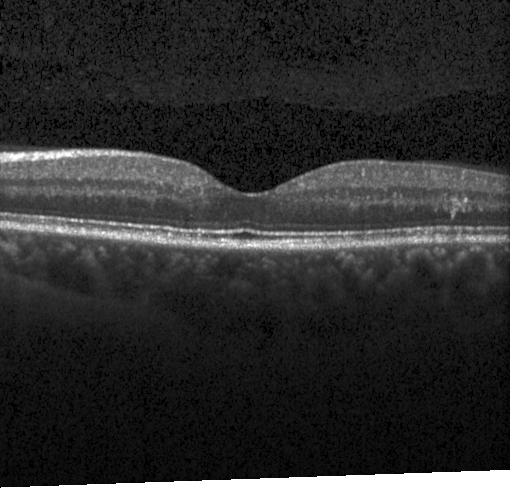
Spectral-domain optical coherence tomography, centered on the fovea, acquired on a Heidelberg Spectralis, OCT line scan — Finding: no evidence of CNV, DME, or drusen.